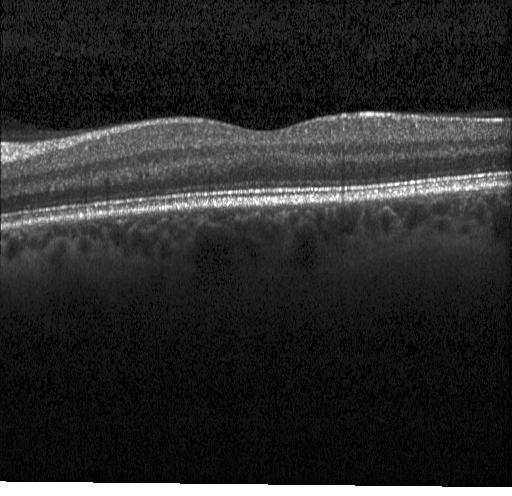 Centered on the fovea. Spectral-domain optical coherence tomography. Optical coherence tomography scan. Heidelberg Spectralis OCT system — Impression: no evidence of CNV, DME, or drusen.